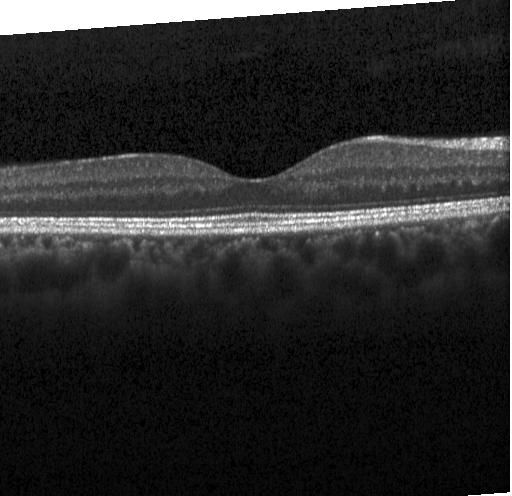

Impression: no evidence of CNV, DME, or drusen.